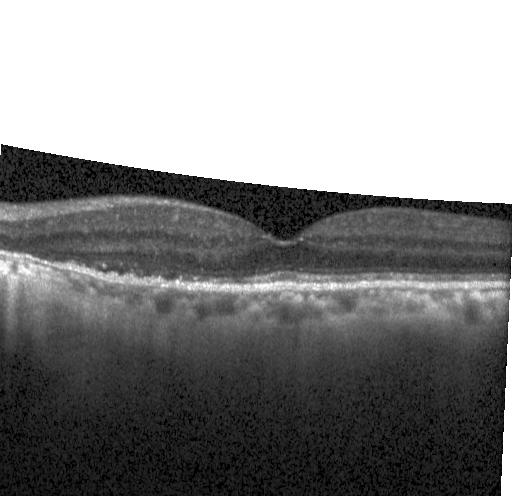
Macular OCT: no CNV, no DME, and no drusen.